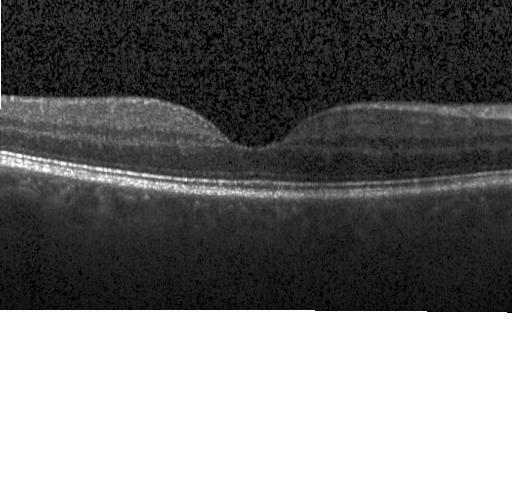
Spectral-domain optical coherence tomography · retinal OCT B-scan — Dx: no evidence of choroidal neovascularization, diabetic macular edema, or drusen.